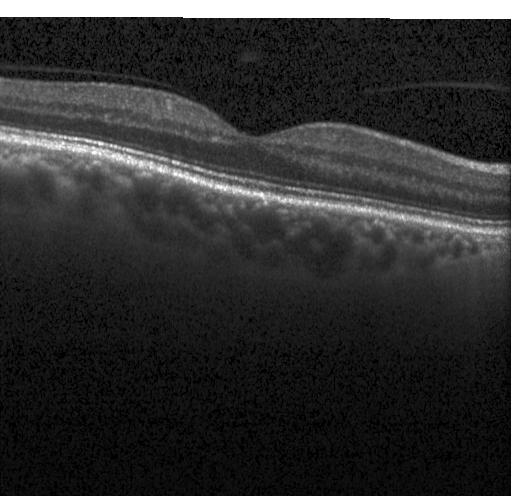

OCT B-scan showing no choroidal neovascularization, diabetic macular edema, or drusen.